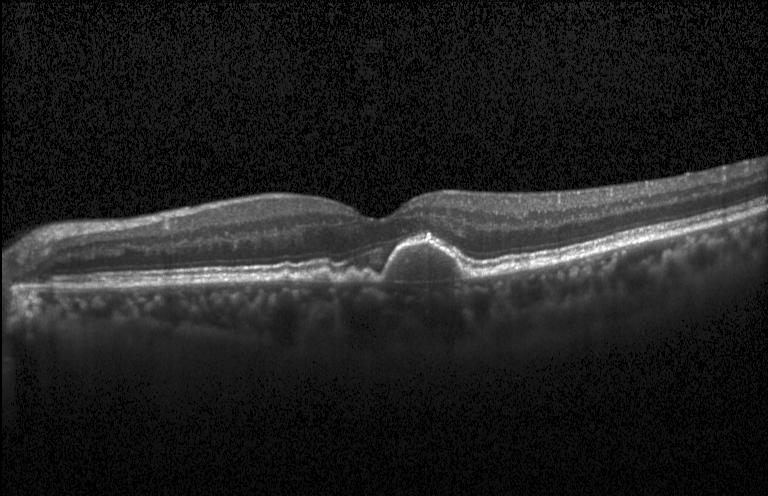
Spectral-domain optical coherence tomography. Retinal OCT cross-section.
Assessment: drusen.